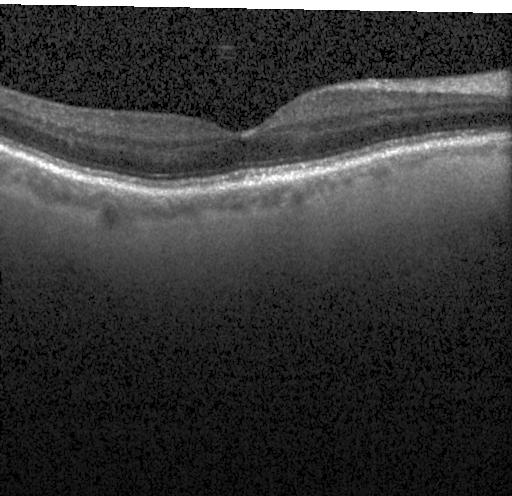

No CNV, DME, or drusen.